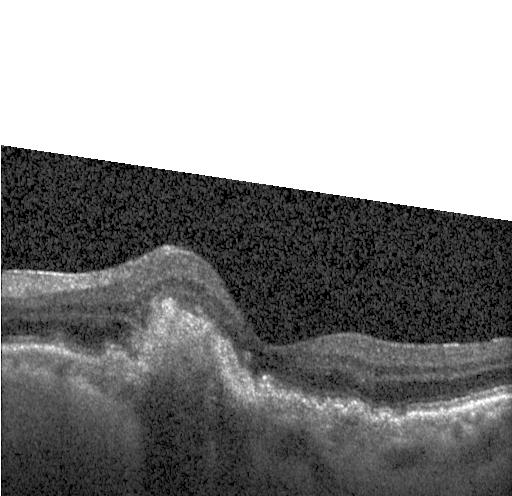
OCT finding: CNV.